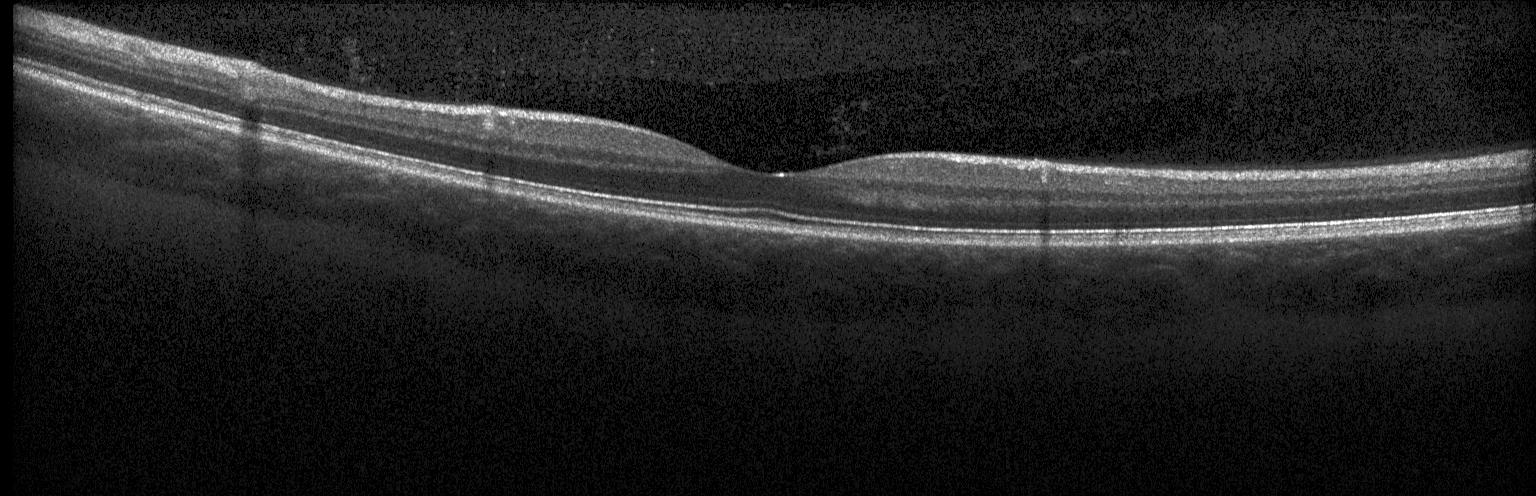
Optical coherence tomography B-scan, Heidelberg Spectralis, through the macula, SD-OCT — Finding: neither CNV, DME, nor drusen.